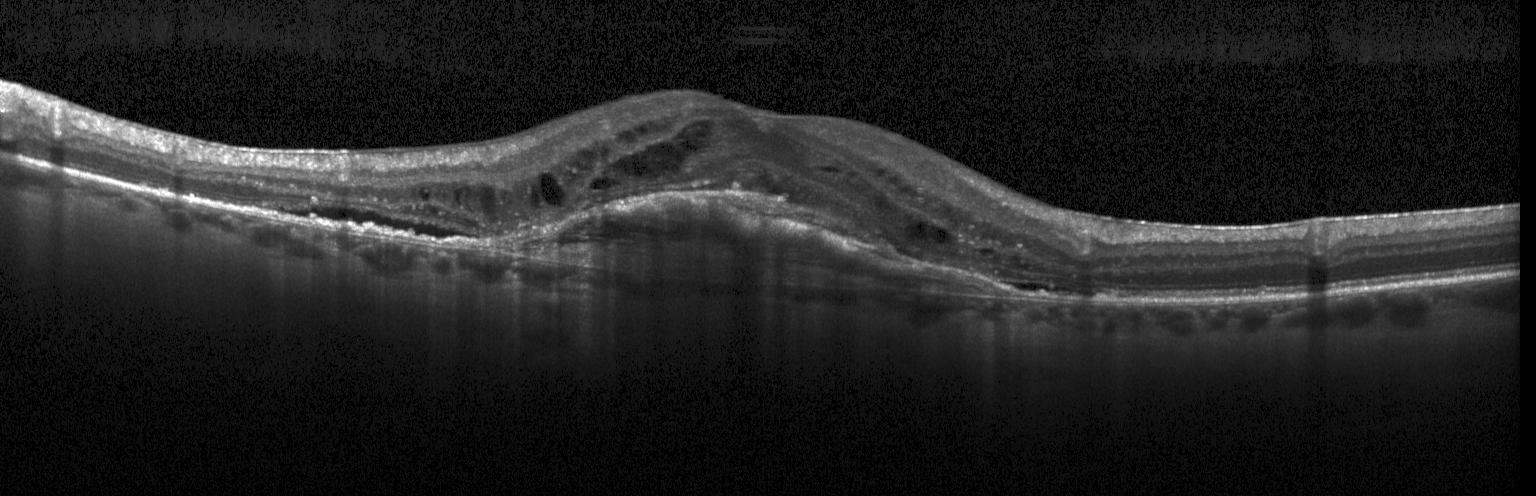
Spectral-domain OCT B-scan: a choroidal neovascular membrane.